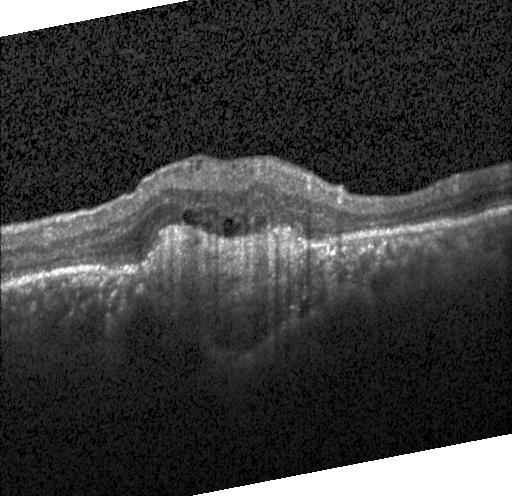
Impression: choroidal neovascularization.